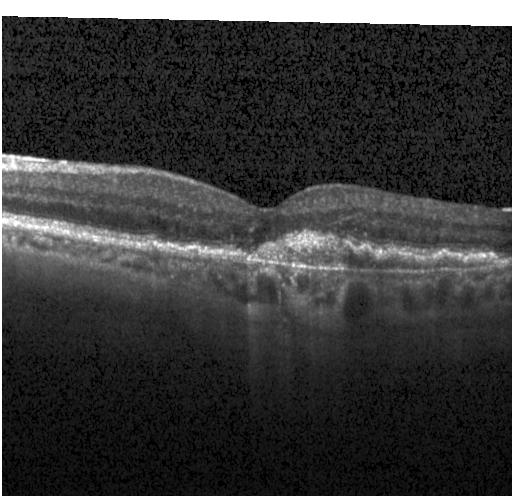
Spectral-domain optical coherence tomography. Centered on the fovea. Acquired on a Heidelberg Spectralis. Optical coherence tomography B-scan — Finding: a choroidal neovascular membrane.